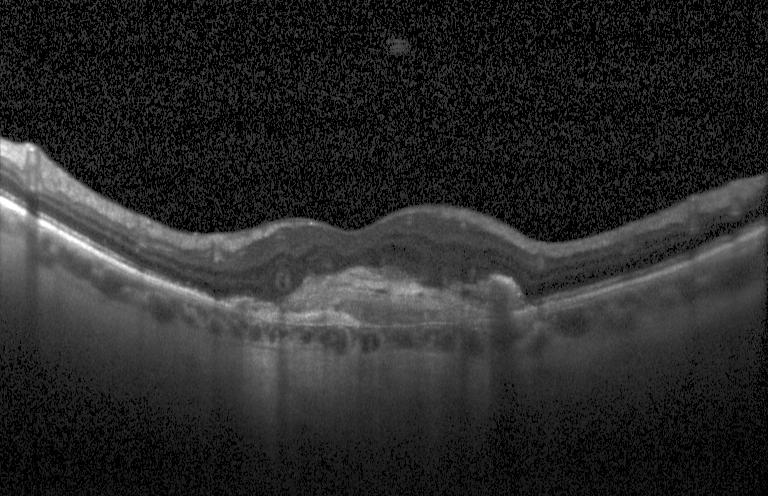
Optical coherence tomography scan. Centered on the fovea.
A choroidal neovascular membrane.